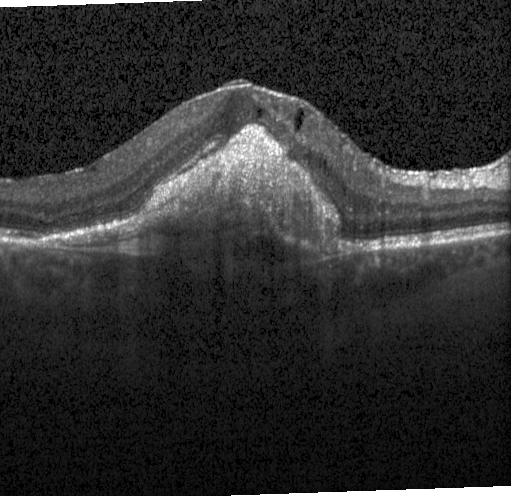
Acquired on a Heidelberg Spectralis, retinal OCT B-scan
Finding: a choroidal neovascular membrane.